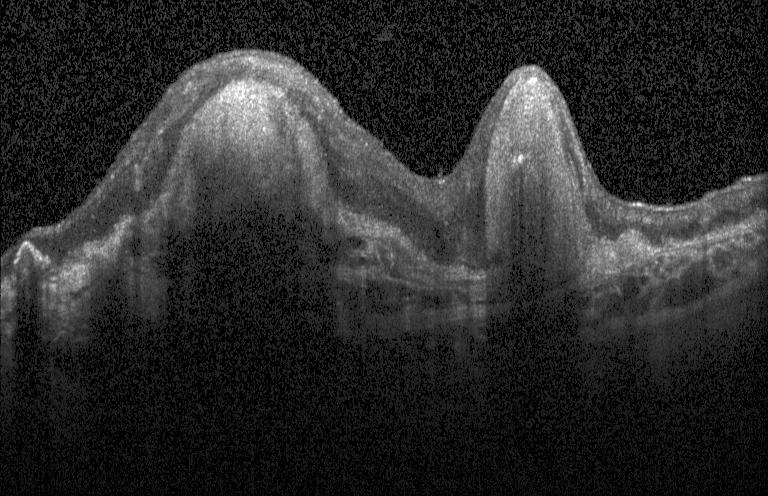

Macular OCT: choroidal neovascularization (CNV).